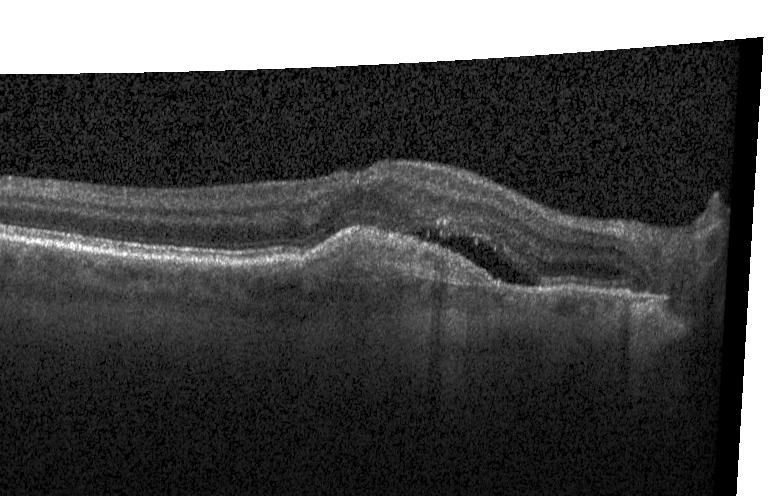

OCT line scan · instrument: Heidelberg Spectralis · through the macula · spectral-domain OCT.
Impression: choroidal neovascularization.